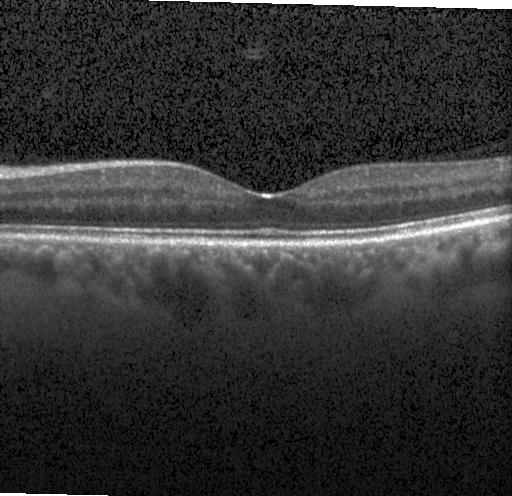 OCT scan showing neither choroidal neovascularization, diabetic macular edema, nor drusen.